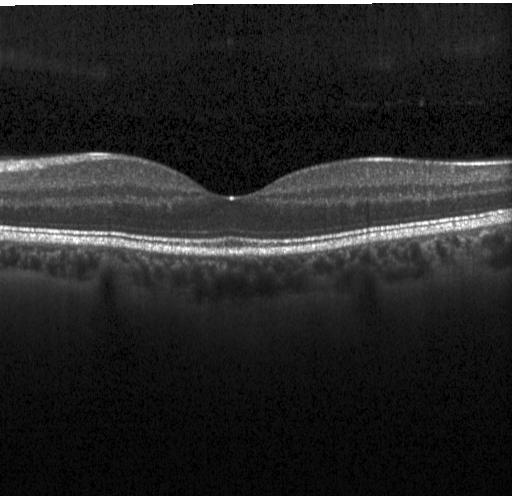

Horizontal scan through the fovea, spectral-domain OCT, instrument: Heidelberg Spectralis, OCT B-scan.
Dx: no choroidal neovascularization, no diabetic macular edema, and no drusen.